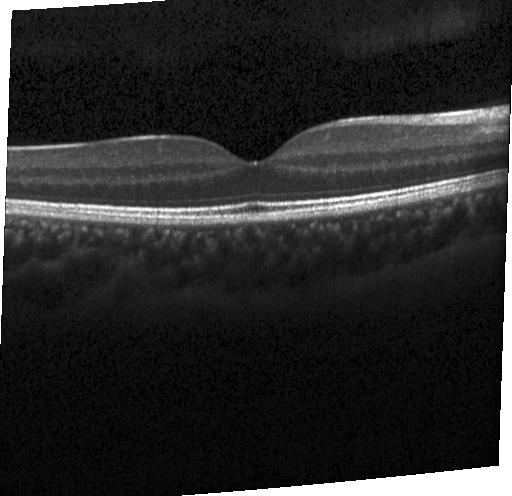 OCT line scan
Impression: no evidence of choroidal neovascularization, diabetic macular edema, or drusen.